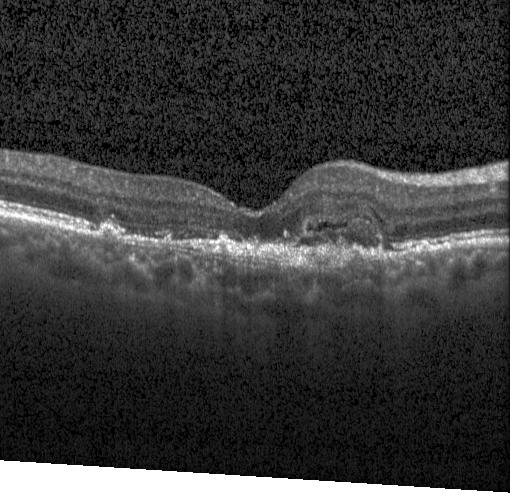 Through the macula · OCT B-scan · Heidelberg Spectralis OCT system · SD-OCT — Dx: CNV.